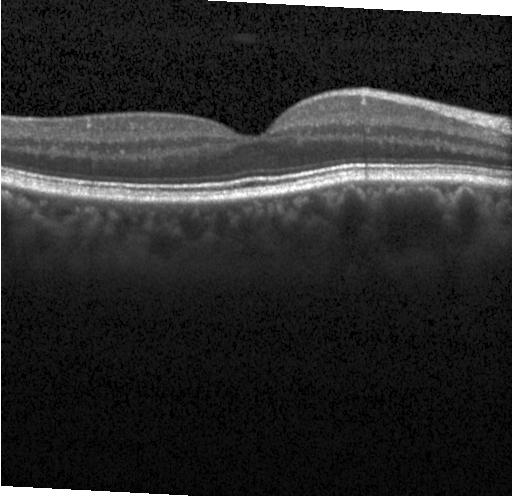 Assessment: no CNV, no DME, and no drusen.